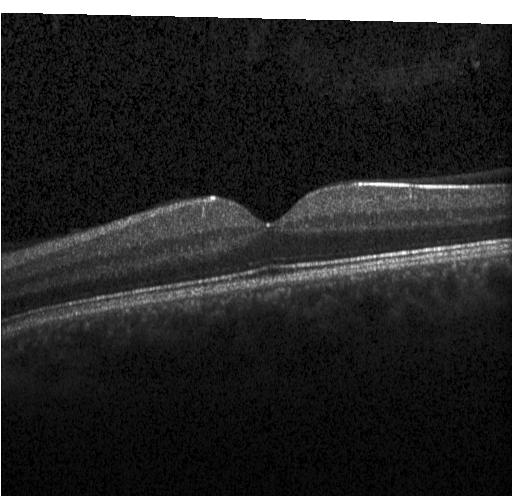

Retinal OCT cross-section. Finding: no CNV, no DME, and no drusen.